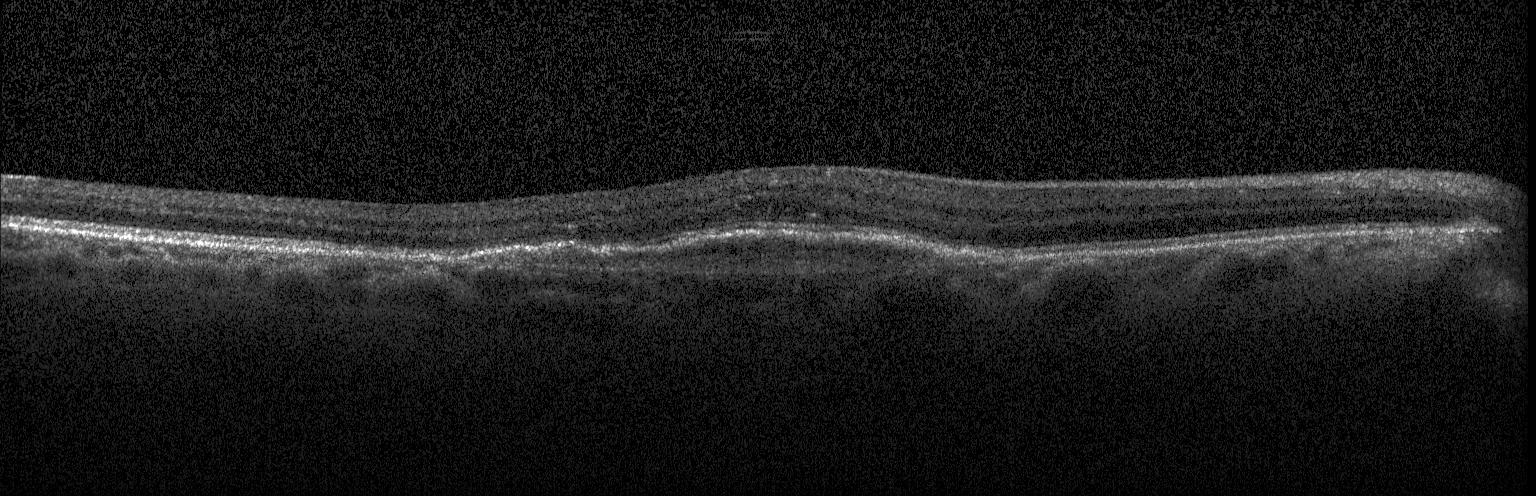 Optical coherence tomography B-scan; acquired on a Heidelberg Spectralis. Finding: a choroidal neovascular membrane.